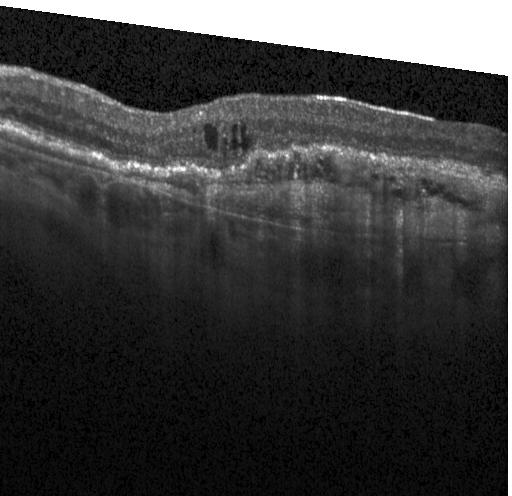

OCT B-scan showing choroidal neovascularization.